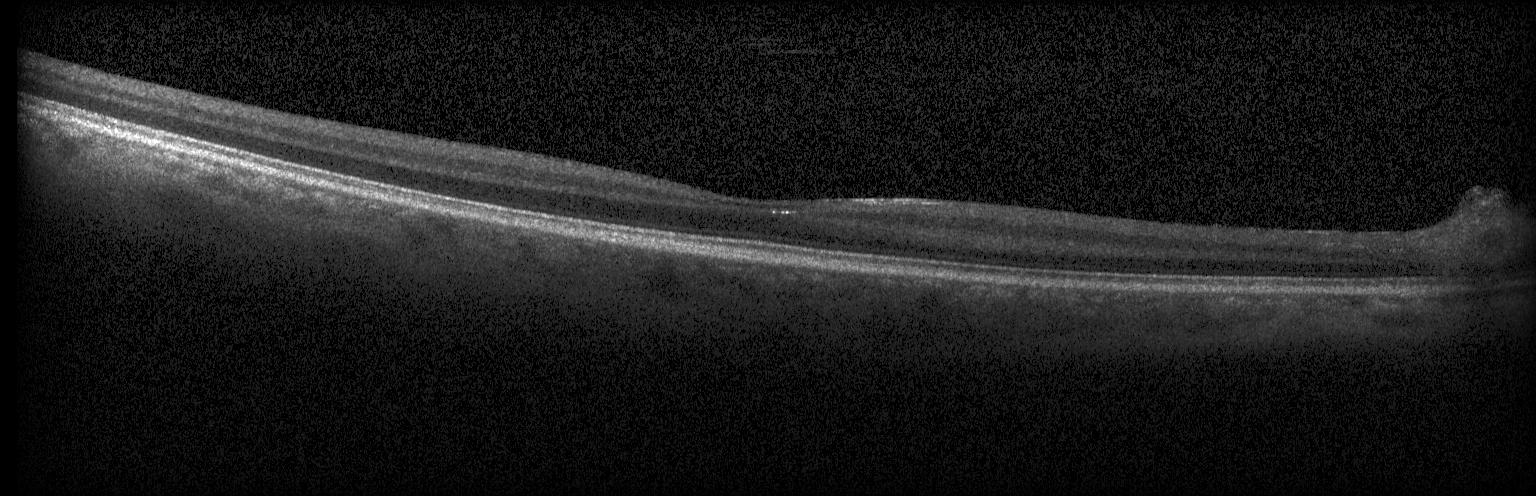

Finding: no evidence of choroidal neovascularization, diabetic macular edema, or drusen.